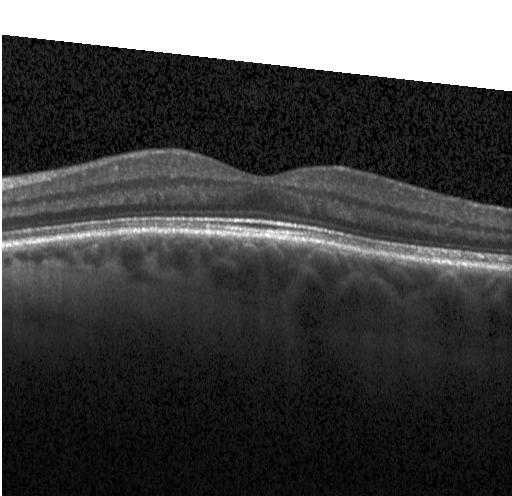 Instrument: Heidelberg Spectralis; optical coherence tomography scan; macular scan; spectral-domain optical coherence tomography — Diagnosis: no choroidal neovascularization, diabetic macular edema, or drusen.